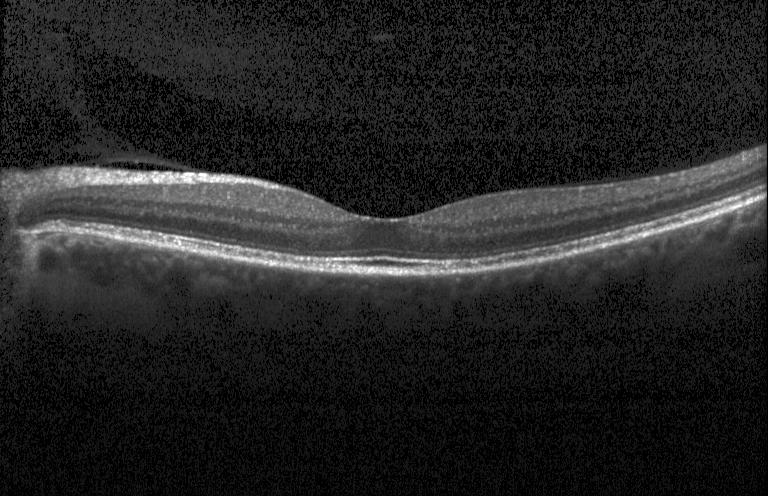 OCT line scan.
Impression: no choroidal neovascularization, no diabetic macular edema, and no drusen.